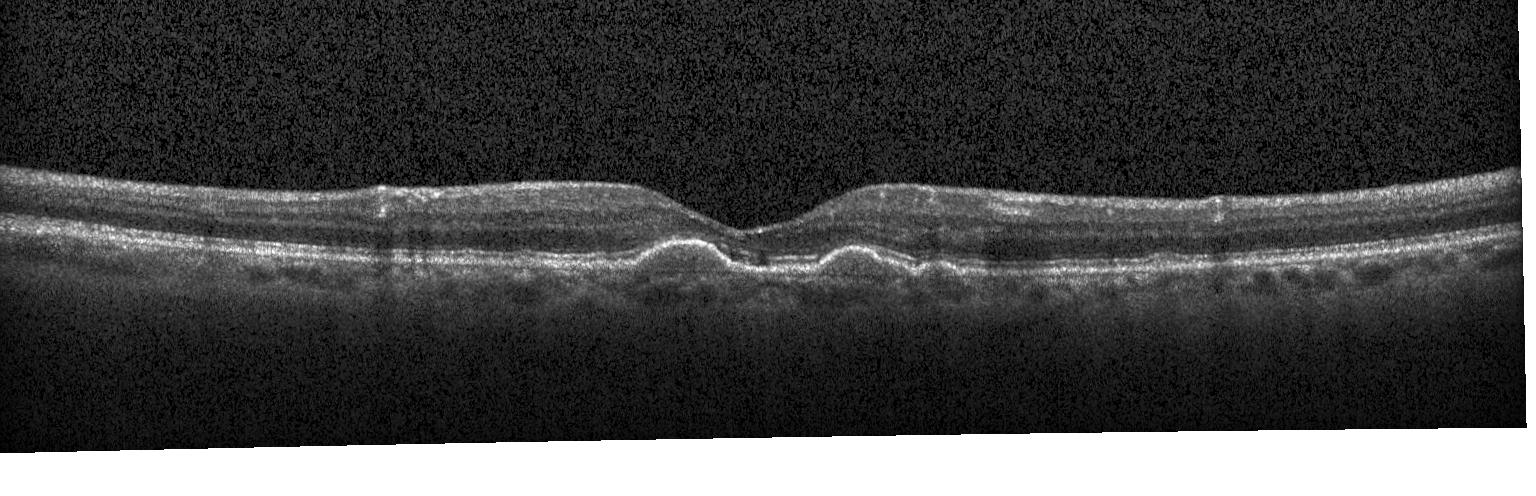 Retinal OCT cross-section; macular scan; acquired on a Heidelberg Spectralis.
This B-scan demonstrates multiple drusen.